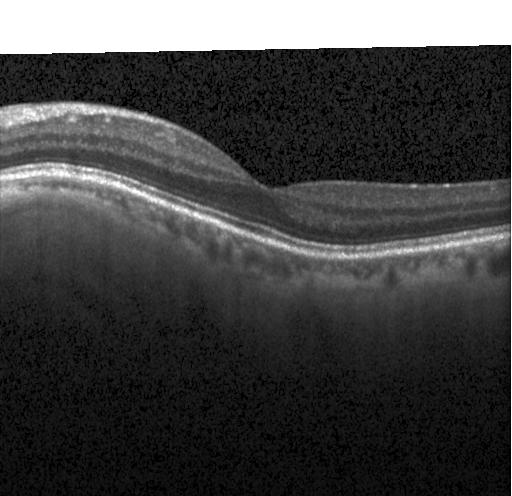
Heidelberg Spectralis OCT system, OCT B-scan — Finding: neither CNV, DME, nor drusen.